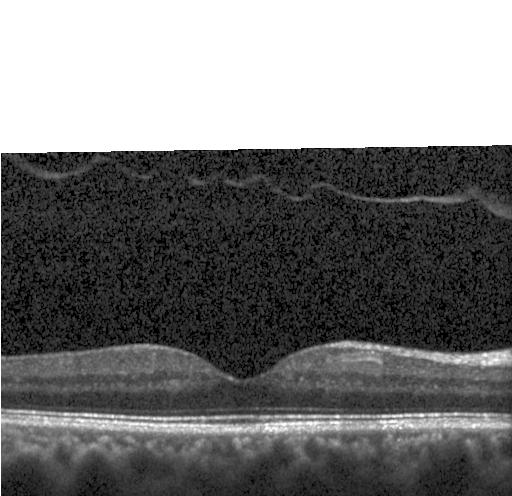 OCT B-scan; macular scan.
The scan shows neither CNV, DME, nor drusen.